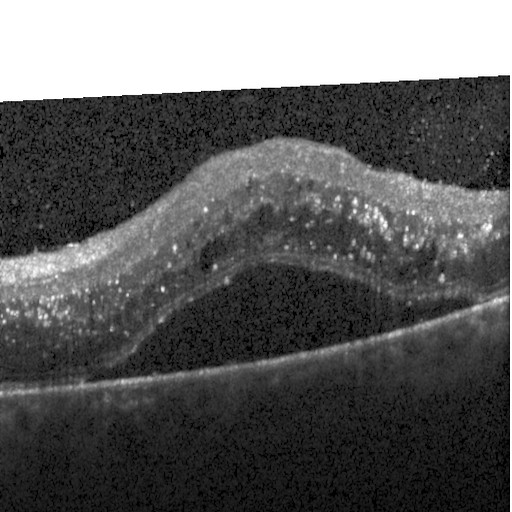 Retinal OCT B-scan. Diagnosis: diabetic macular edema (DME).